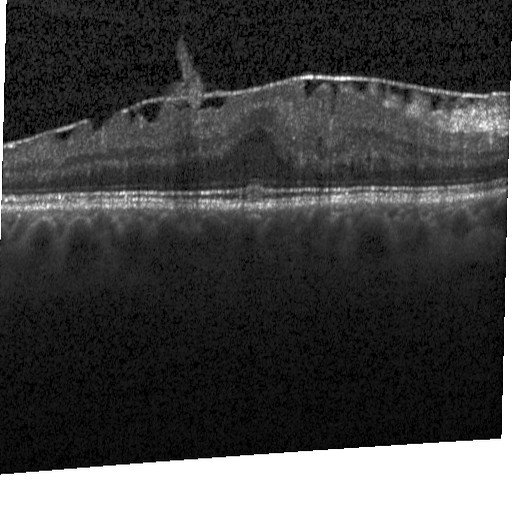 OCT line scan, fovea-centered. Diabetic macular edema.